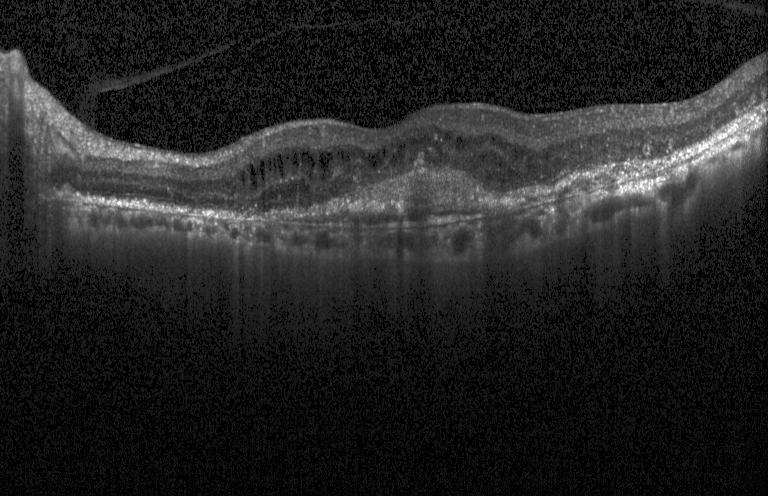
Spectral-domain OCT · optical coherence tomography scan. This B-scan demonstrates CNV.